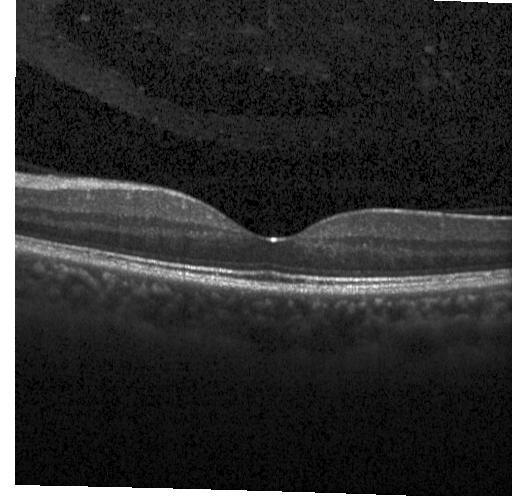
Optical coherence tomography B-scan. Assessment: neither CNV, DME, nor drusen.